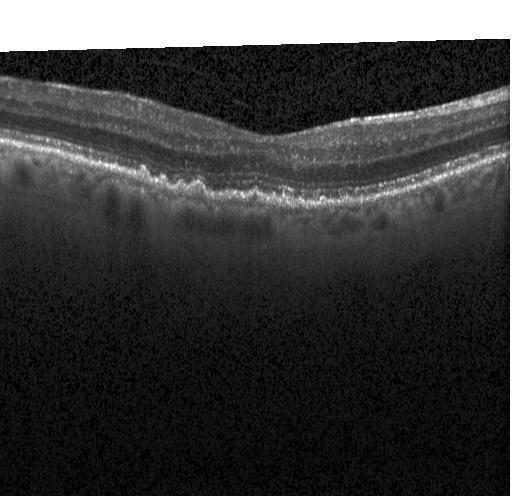 Macular OCT demonstrating drusen.